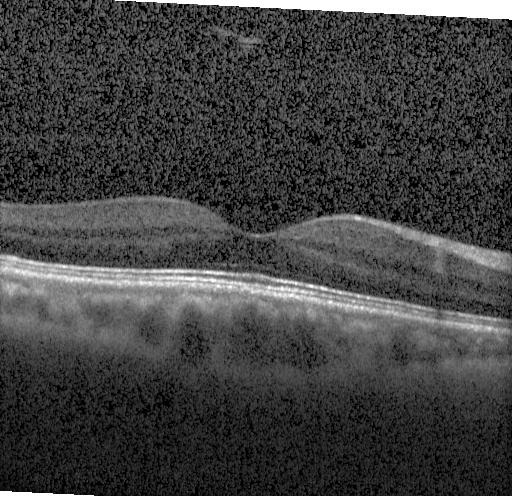

Instrument: Heidelberg Spectralis, fovea-centered, OCT line scan
This B-scan demonstrates no CNV, DME, or drusen.